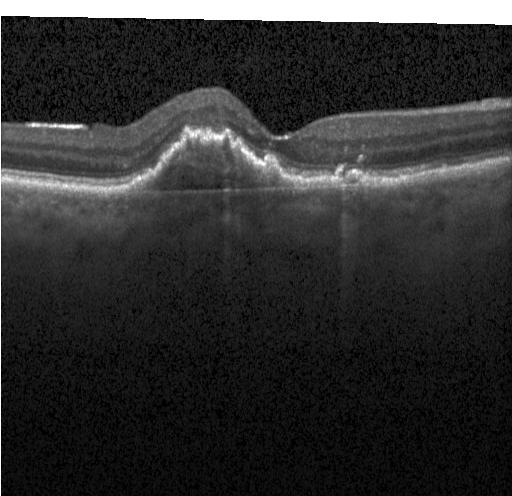
Finding: a choroidal neovascular membrane.